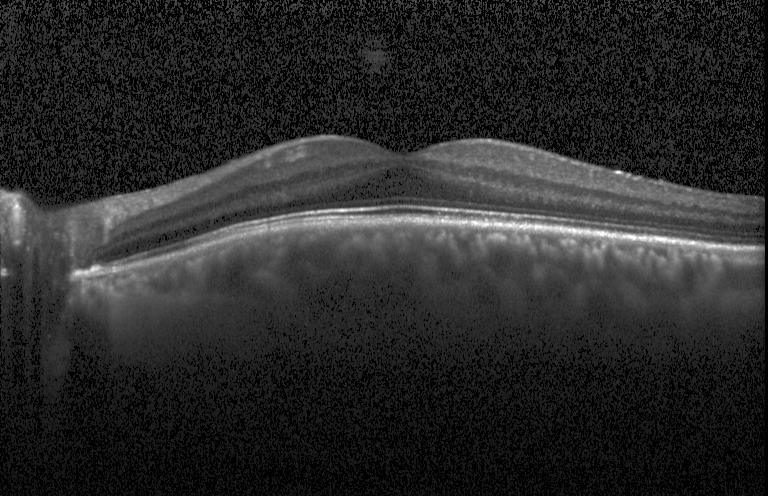 No CNV, DME, or drusen.